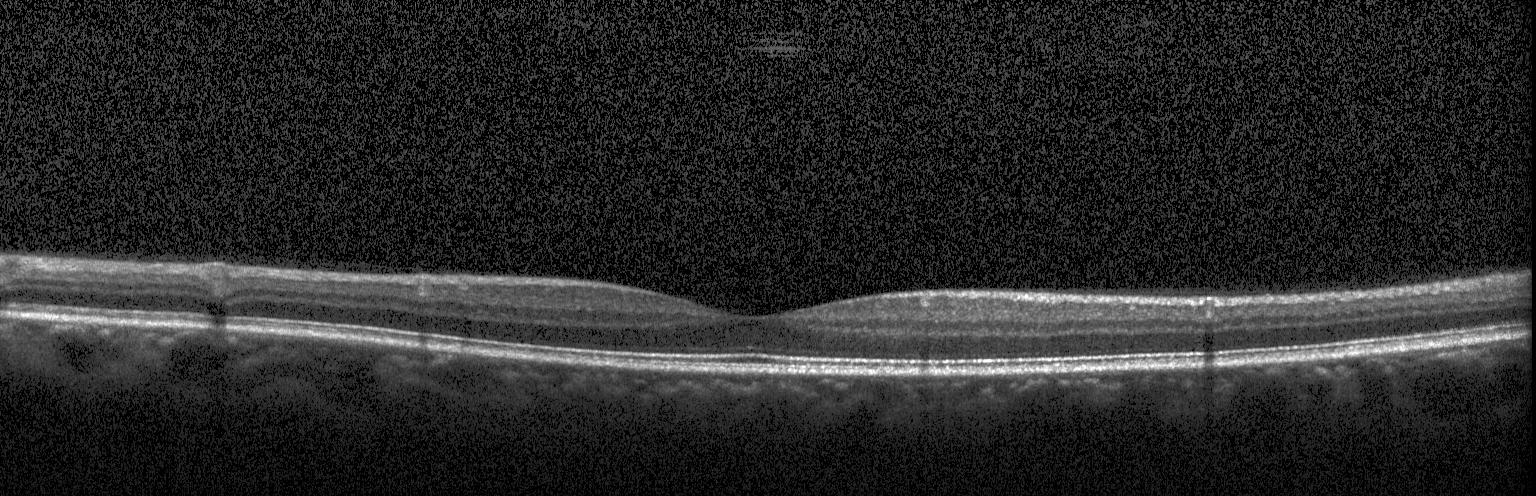 Spectral-domain optical coherence tomography · horizontal scan through the fovea · OCT B-scan — Finding: no choroidal neovascularization, no diabetic macular edema, and no drusen.